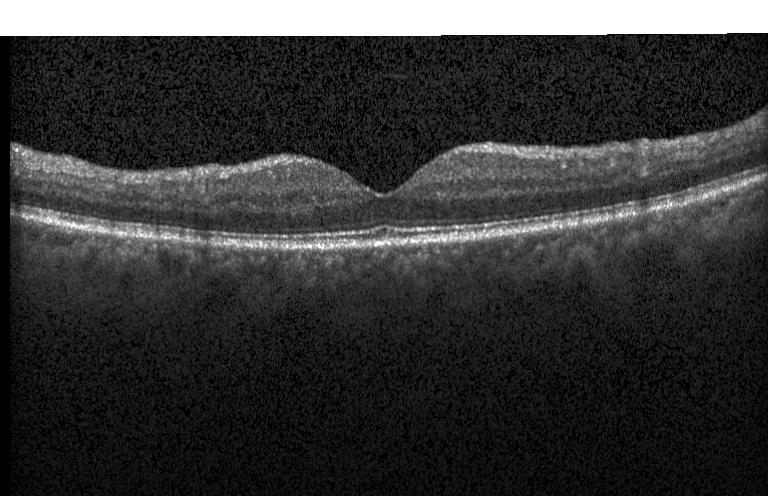
OCT scan showing no choroidal neovascularization, diabetic macular edema, or drusen.